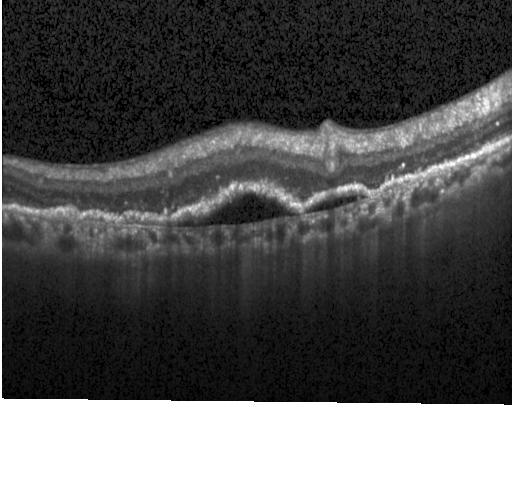 Spectral-domain OCT B-scan: CNV.